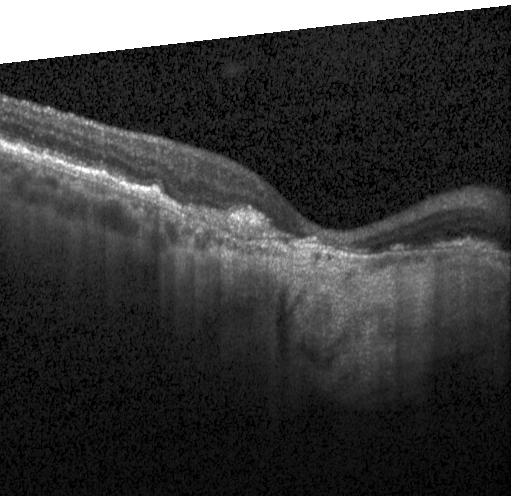

Through the macula. SD-OCT. OCT B-scan. Instrument: Heidelberg Spectralis — Macular OCT: a choroidal neovascular membrane.